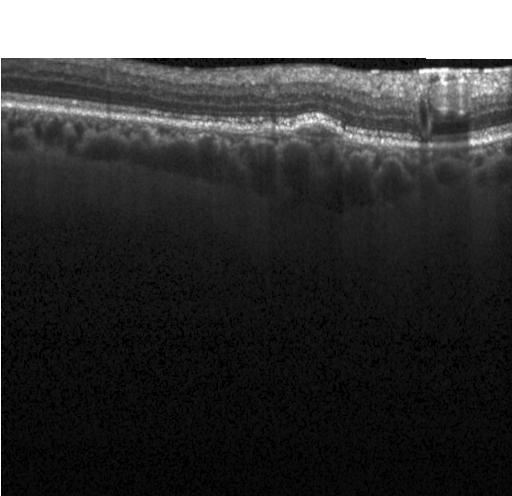 Macular scan, OCT line scan. Finding: sub-RPE drusenoid deposits.